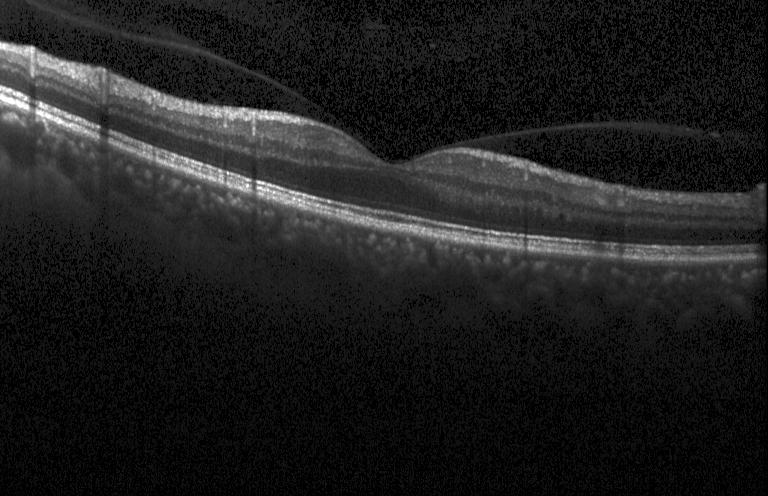

Macular OCT: no choroidal neovascularization, diabetic macular edema, or drusen.